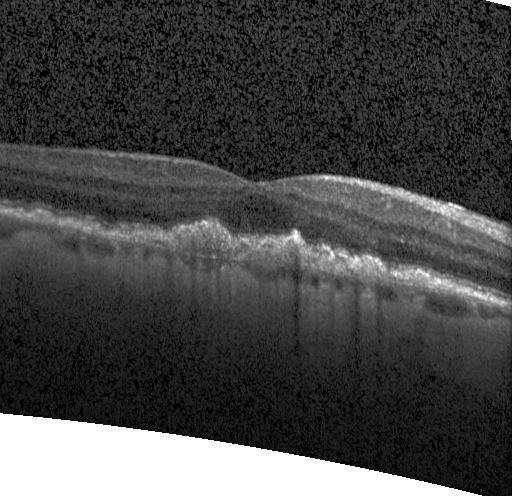

Retinal OCT B-scan; horizontal scan through the fovea — Diagnosis: a choroidal neovascular membrane.